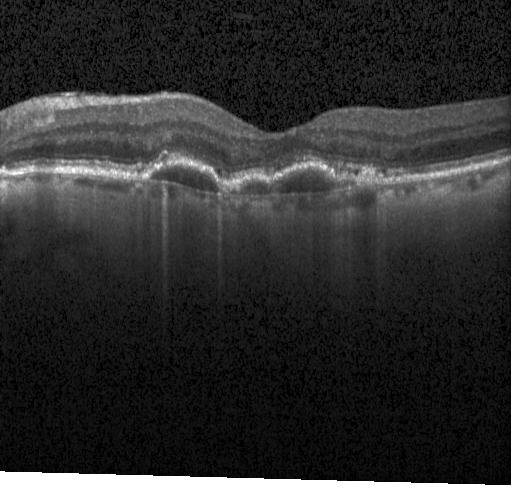 OCT finding: a choroidal neovascular membrane.